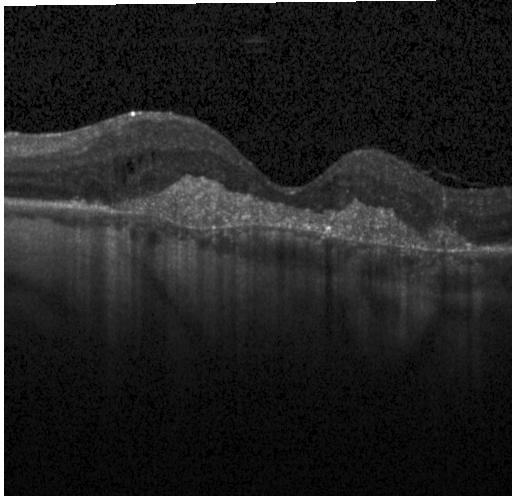 Through the macula · SD-OCT · retinal OCT B-scan.
Macular OCT: a choroidal neovascular membrane.